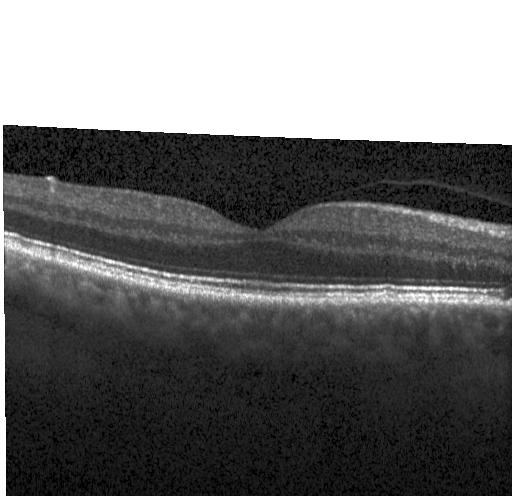 Macular scan. OCT line scan. Impression: no CNV, DME, or drusen.